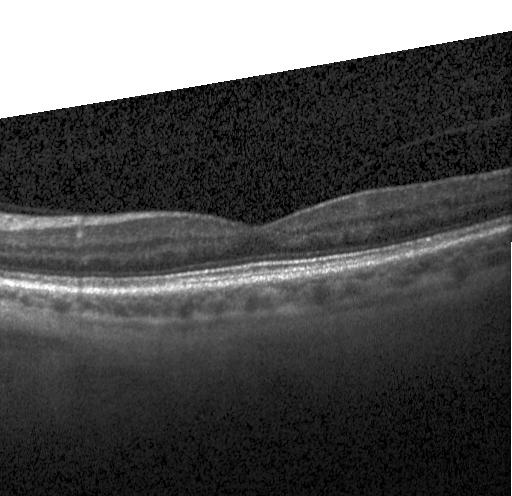 Instrument: Heidelberg Spectralis. Horizontal scan through the fovea. Optical coherence tomography B-scan. Spectral-domain OCT.
Finding: no choroidal neovascularization, diabetic macular edema, or drusen.